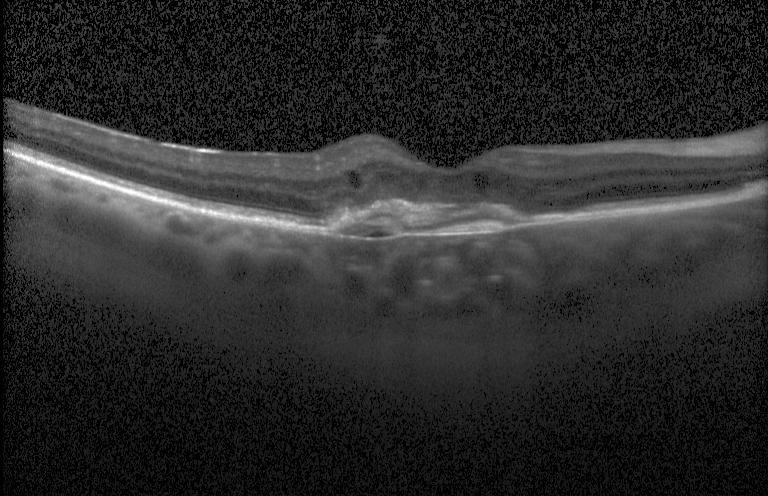 Impression: choroidal neovascularization (CNV).